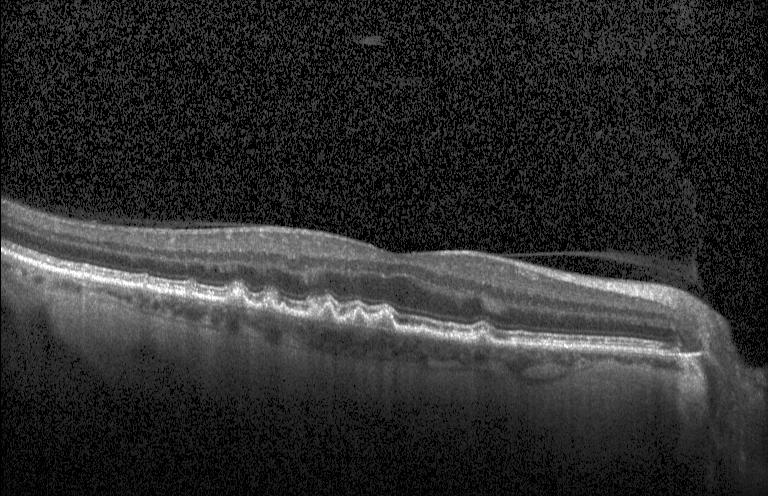
Spectral-domain optical coherence tomography. Retinal OCT B-scan.
OCT finding: drusen.